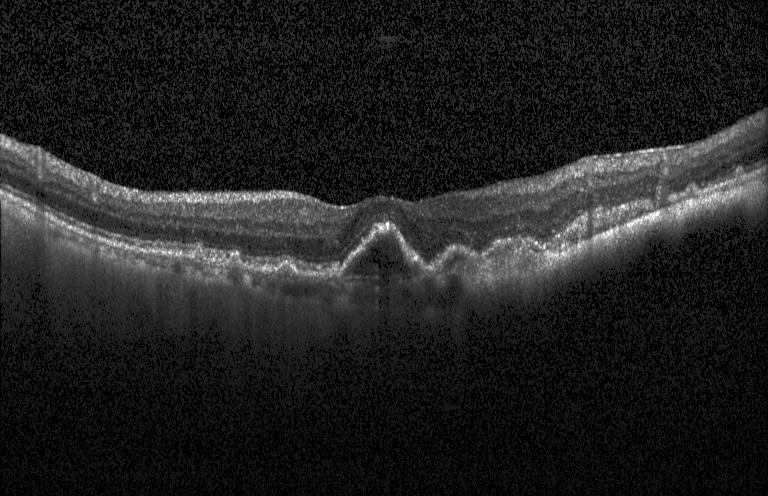

Finding: a choroidal neovascular membrane.